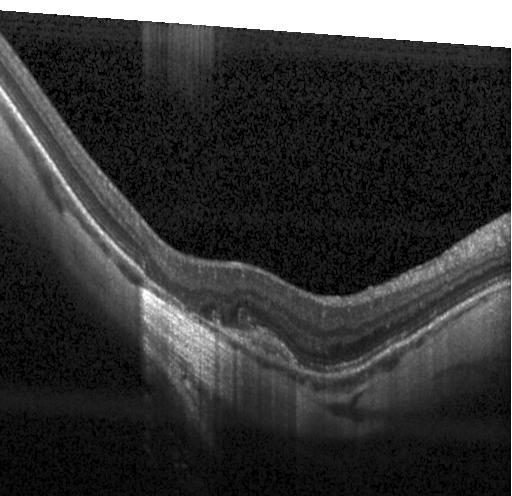 Optical coherence tomography B-scan, centered on the fovea, instrument: Heidelberg Spectralis, SD-OCT. Diagnosis: a choroidal neovascular membrane.